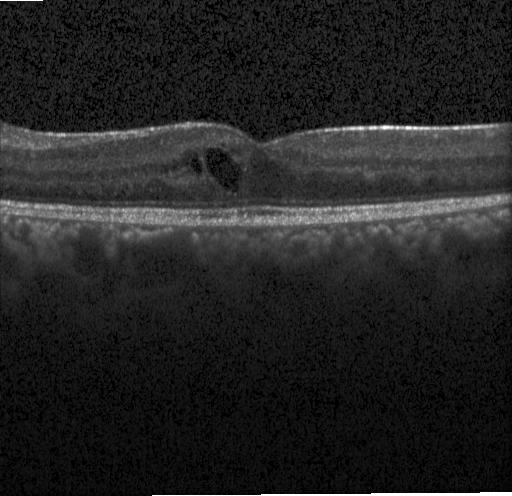

Macular OCT: diabetic macular edema.